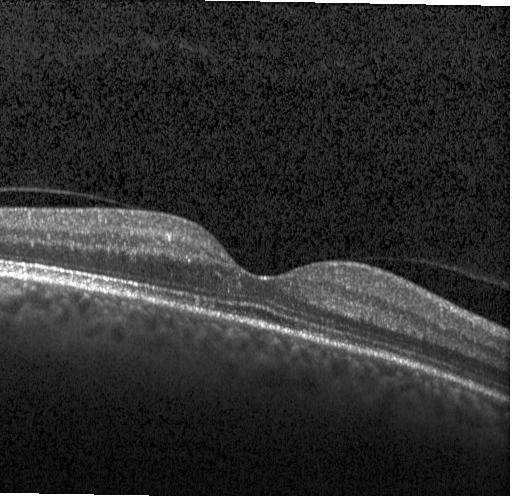
No evidence of CNV, DME, or drusen.